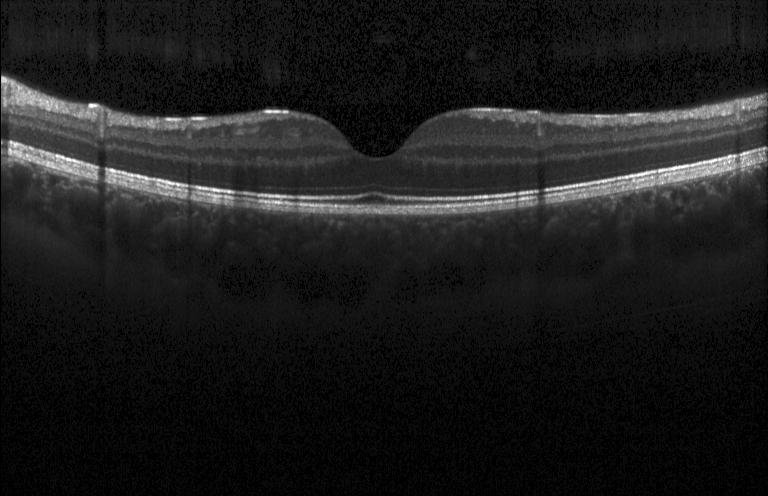 Optical coherence tomography scan, horizontal scan through the fovea, SD-OCT, Heidelberg Spectralis OCT system.
Assessment: neither choroidal neovascularization, diabetic macular edema, nor drusen.